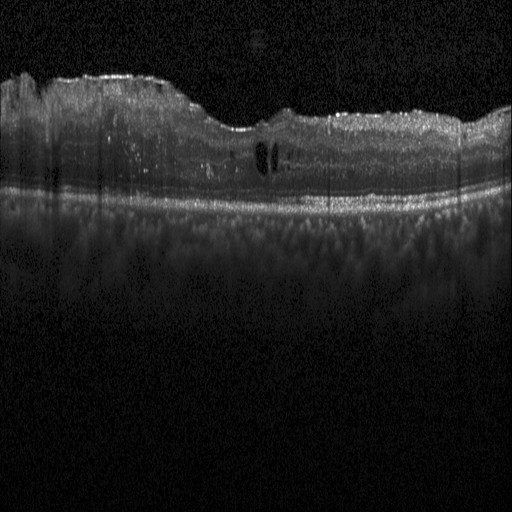

Finding: DME.